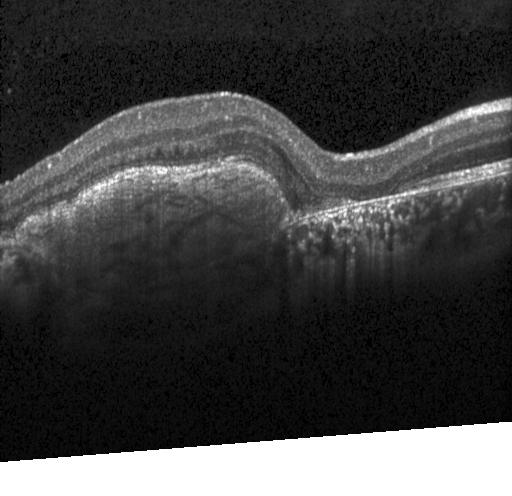
Retinal OCT B-scan
Impression: a choroidal neovascular membrane.